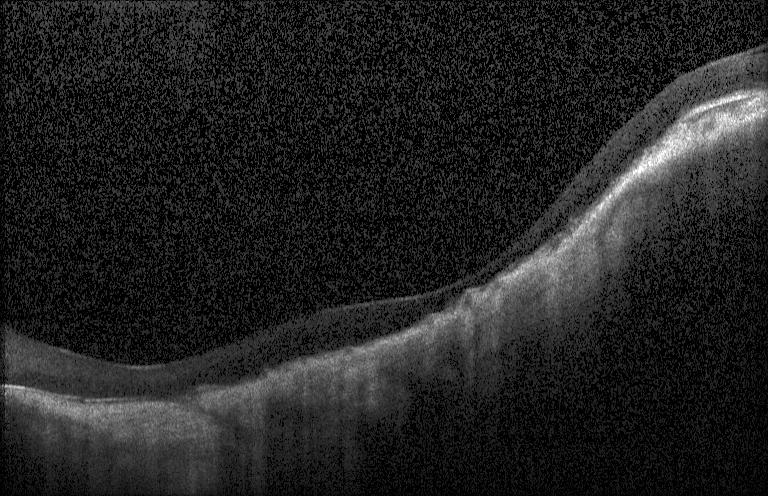 Acquired on a Heidelberg Spectralis, OCT line scan.
Impression: a choroidal neovascular membrane.